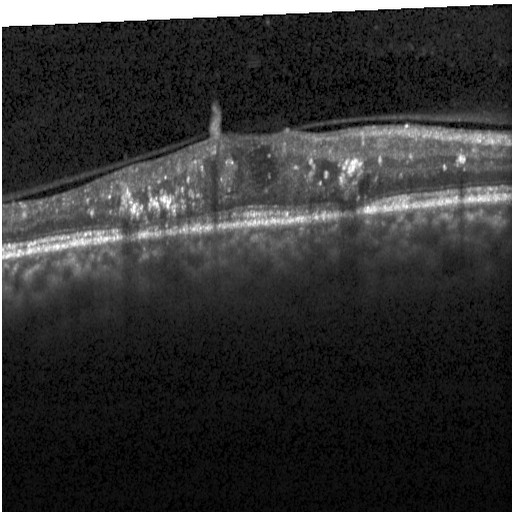 Optical coherence tomography scan · spectral-domain optical coherence tomography
OCT finding: diabetic macular edema (DME).